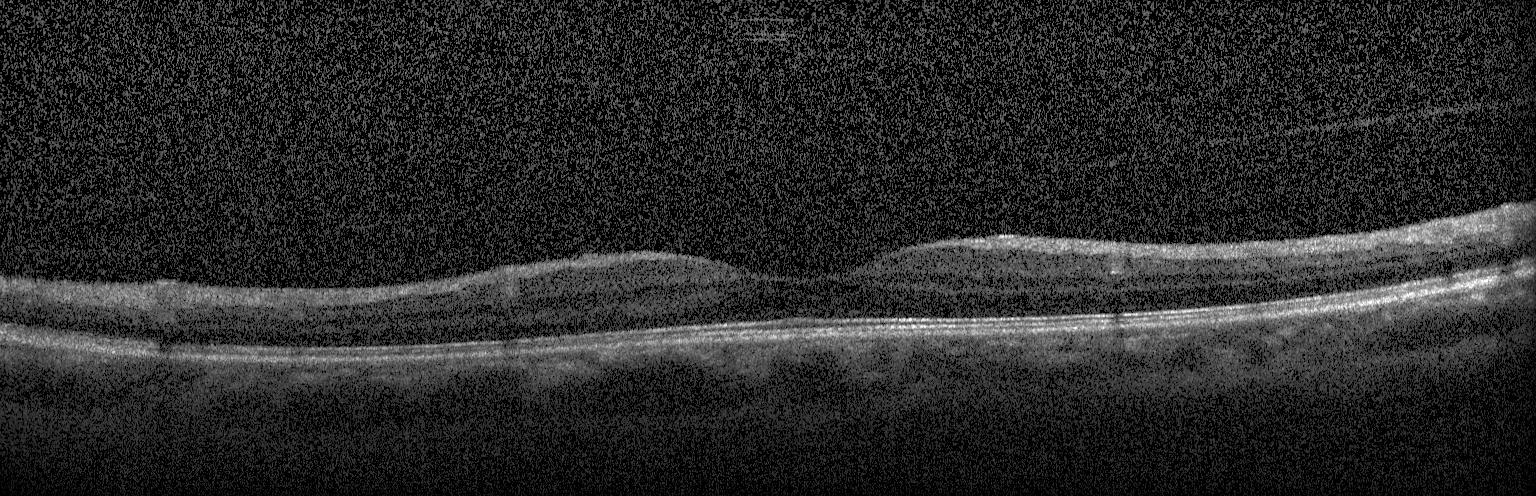

Optical coherence tomography scan
The scan shows neither CNV, DME, nor drusen.